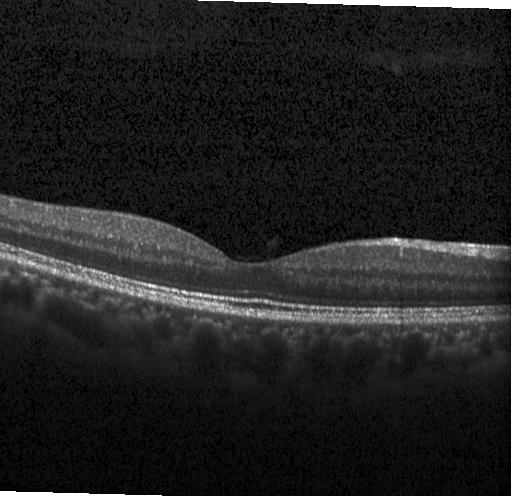

Spectral-domain OCT, Heidelberg Spectralis, OCT line scan, horizontal scan through the fovea. Impression: no evidence of choroidal neovascularization, diabetic macular edema, or drusen.